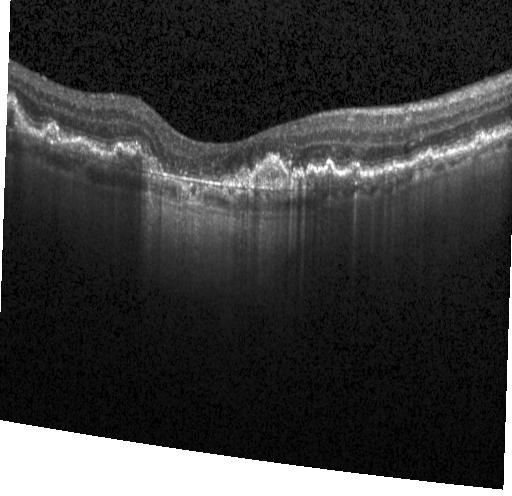

OCT scan showing choroidal neovascularization (CNV).